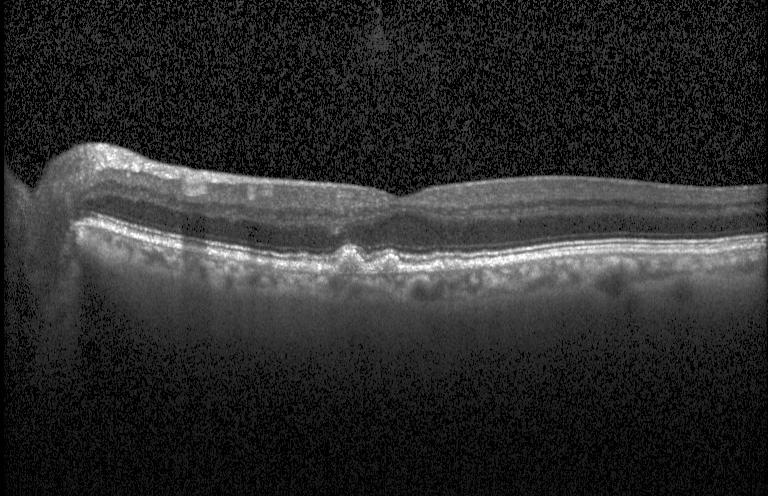 Retinal OCT cross-section.
Finding: drusen.